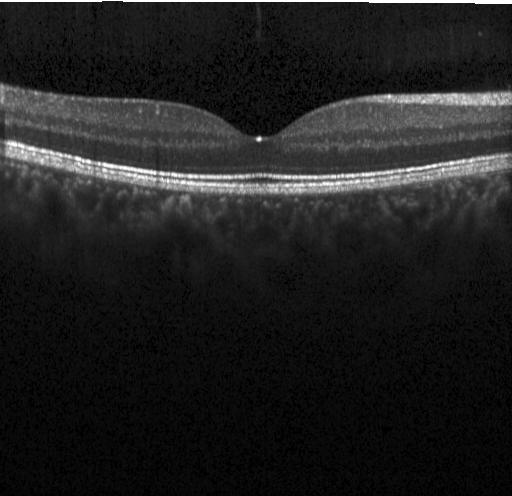
Horizontal scan through the fovea · spectral-domain optical coherence tomography · optical coherence tomography B-scan · instrument: Heidelberg Spectralis
Diagnosis: no choroidal neovascularization, no diabetic macular edema, and no drusen.